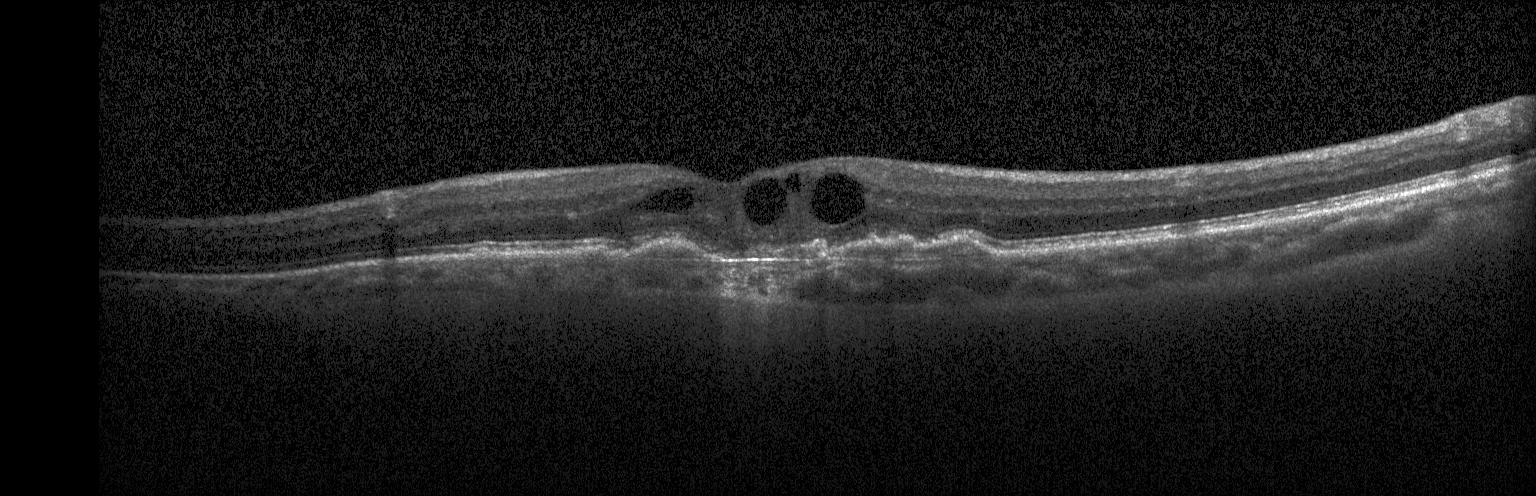 Retinal OCT cross-section showing a choroidal neovascular membrane.